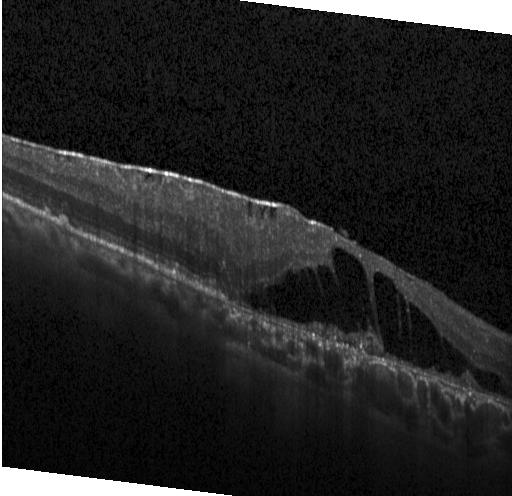

OCT line scan · macular scan
Diagnosis: a choroidal neovascular membrane.